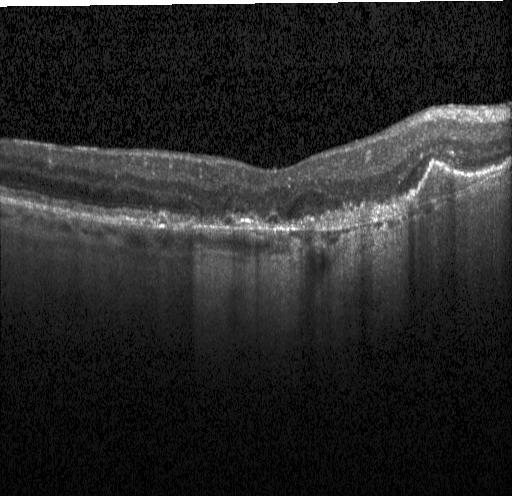 Through the macula; SD-OCT; retinal OCT B-scan — Macular OCT: a choroidal neovascular membrane.